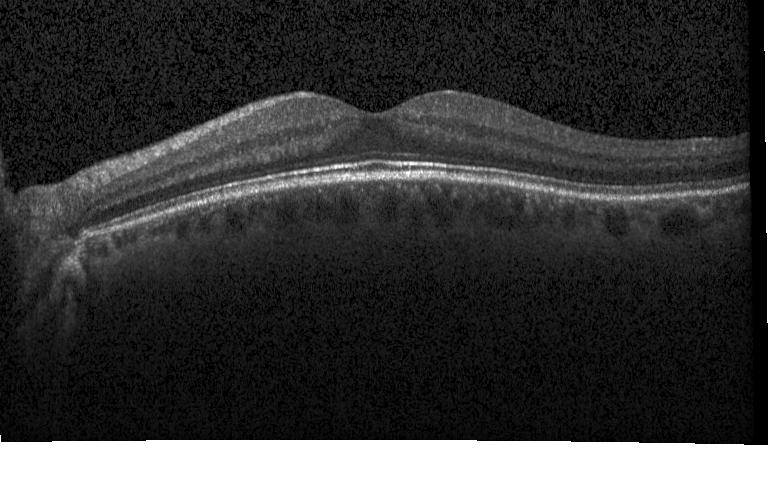
Spectral-domain optical coherence tomography, macular scan, retinal OCT B-scan. Dx: neither choroidal neovascularization, diabetic macular edema, nor drusen.